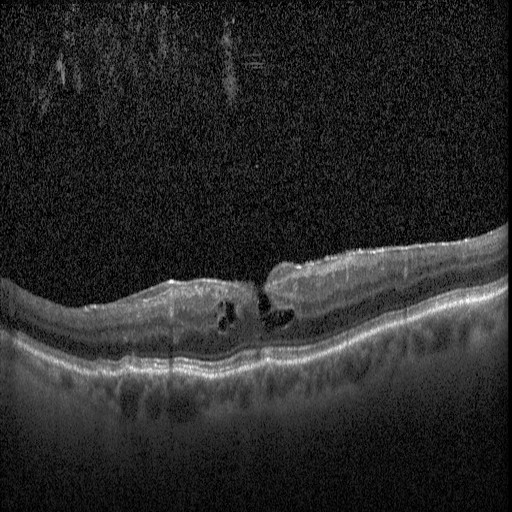 OCT B-scan; spectral-domain optical coherence tomography; instrument: Heidelberg Spectralis; centered on the fovea
Assessment: diabetic macular edema.